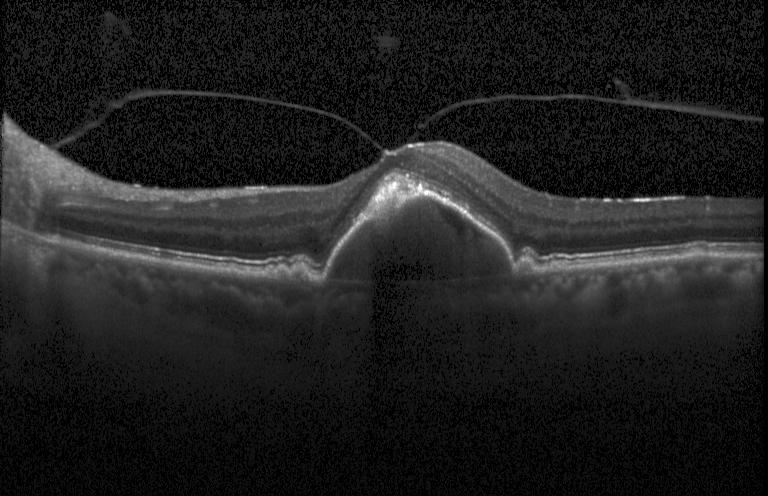 Diagnosis: CNV.